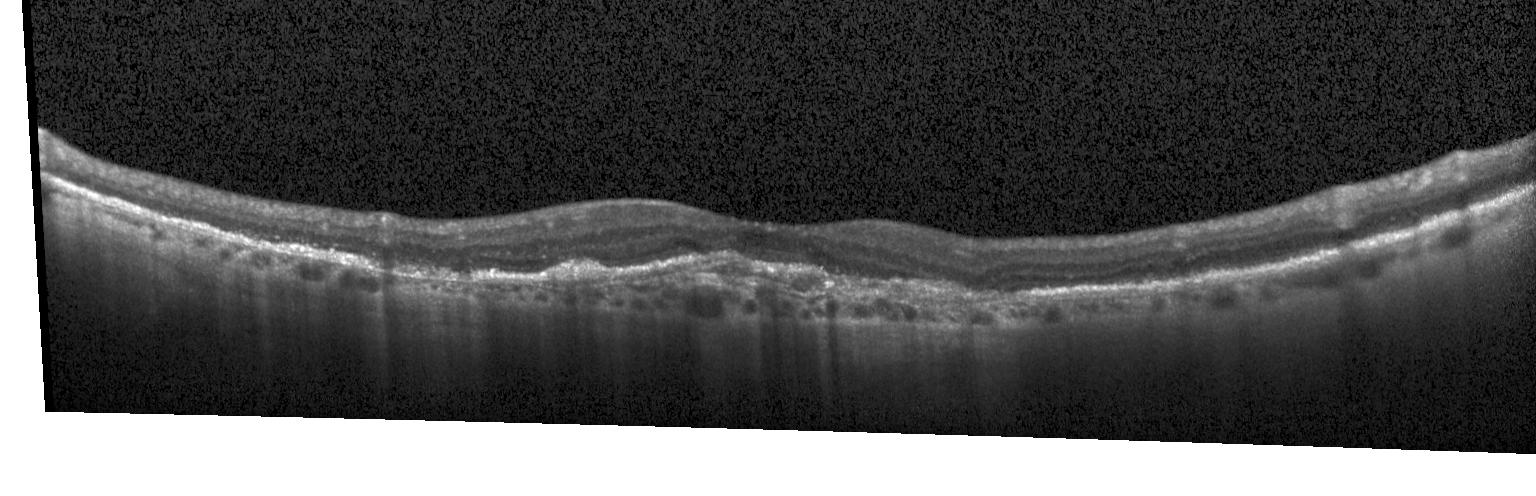

Optical coherence tomography scan. Spectral-domain OCT. Centered on the fovea. Heidelberg Spectralis
Impression: choroidal neovascularization (CNV).